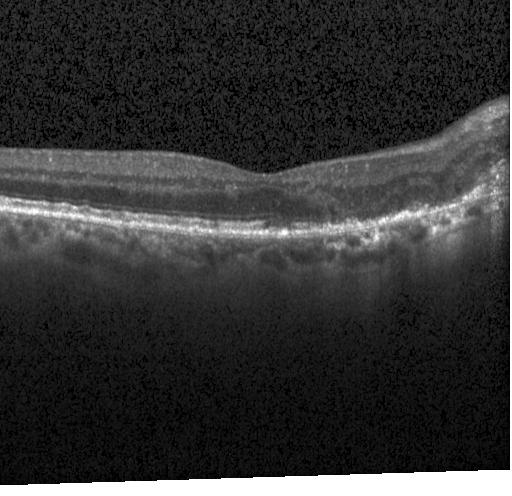 Instrument: Heidelberg Spectralis · fovea-centered · spectral-domain optical coherence tomography · OCT line scan
Diagnosis: a choroidal neovascular membrane.